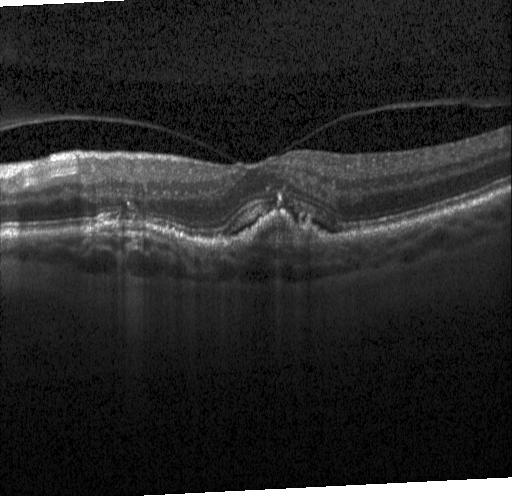

SD-OCT; OCT line scan; horizontal scan through the fovea. OCT finding: a choroidal neovascular membrane.